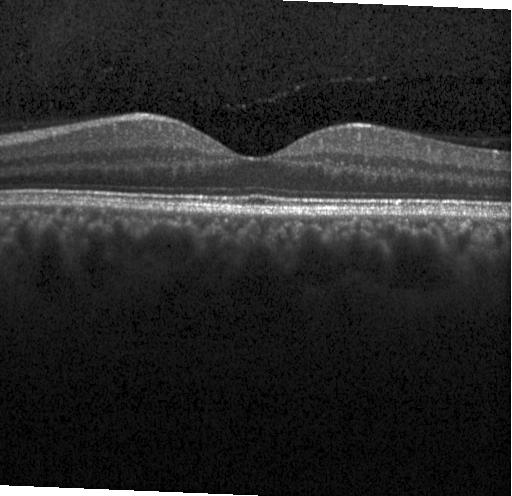
Fovea-centered, spectral-domain optical coherence tomography, OCT line scan — Diagnosis: no choroidal neovascularization, diabetic macular edema, or drusen.